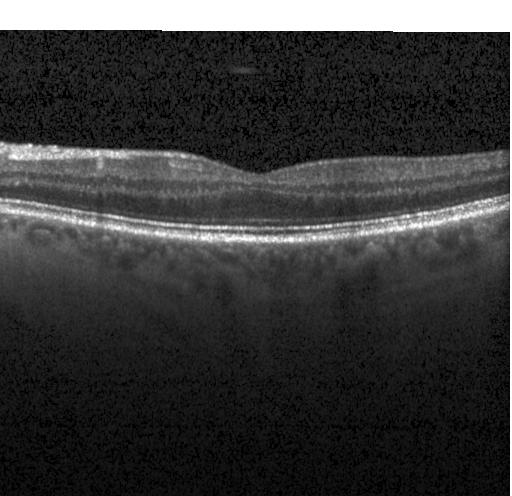

Impression: no choroidal neovascularization, diabetic macular edema, or drusen.